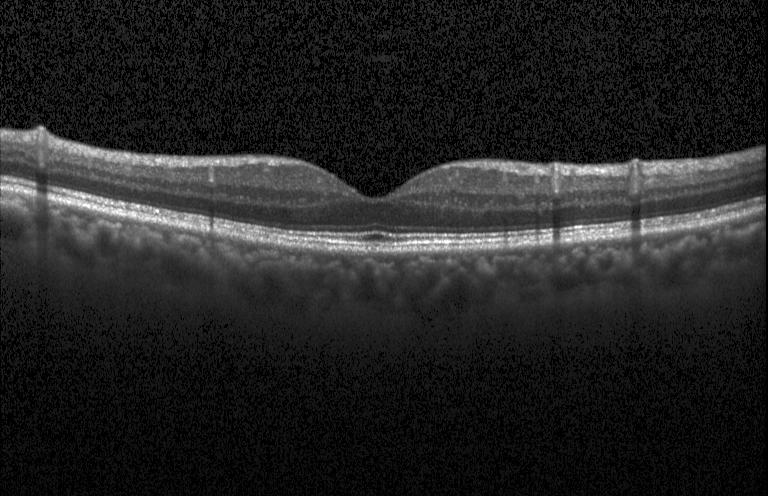

SD-OCT, fovea-centered, optical coherence tomography B-scan
Finding: neither CNV, DME, nor drusen.